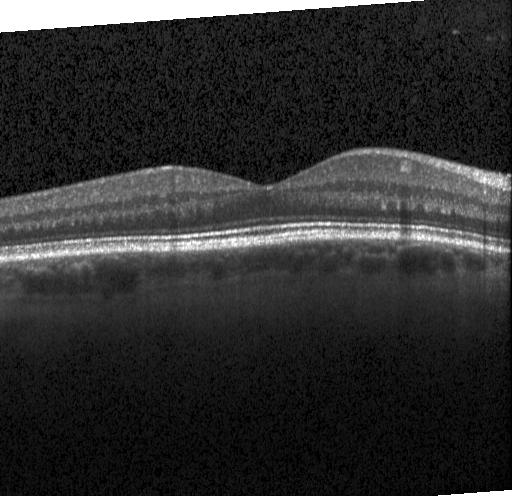 Impression: neither CNV, DME, nor drusen.